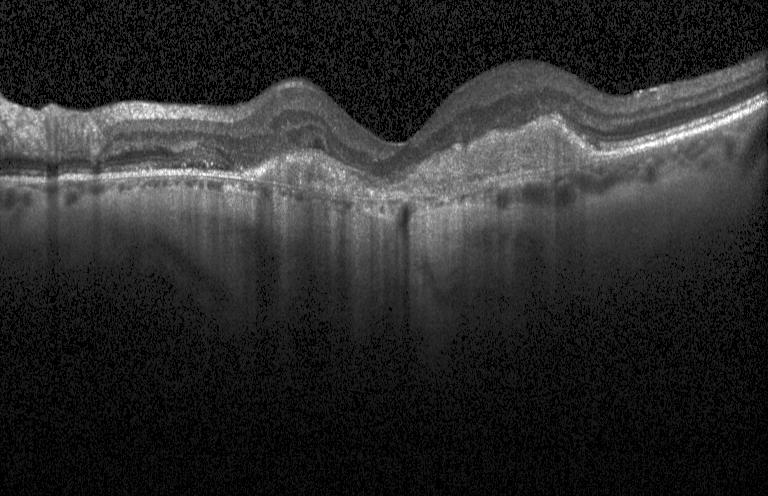
Spectral-domain optical coherence tomography · retinal OCT cross-section · Heidelberg Spectralis — Finding: CNV.